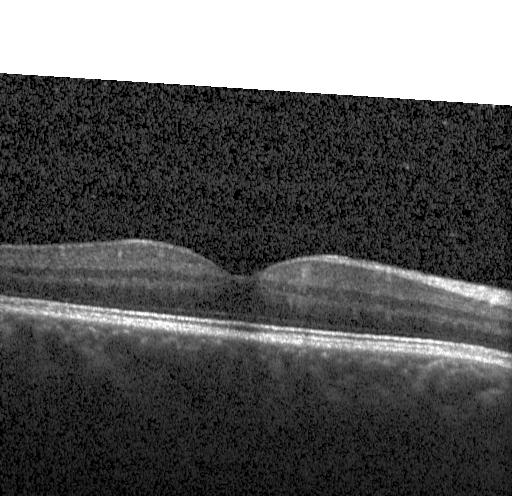
Horizontal scan through the fovea, spectral-domain OCT, retinal OCT cross-section
No evidence of choroidal neovascularization, diabetic macular edema, or drusen.